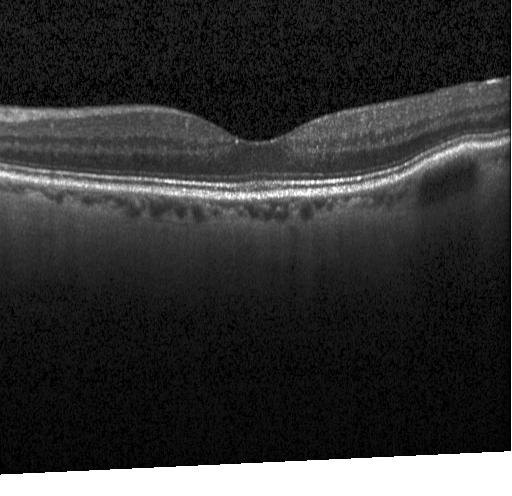

Acquired on a Heidelberg Spectralis. Optical coherence tomography B-scan. Horizontal scan through the fovea. Finding: neither CNV, DME, nor drusen.